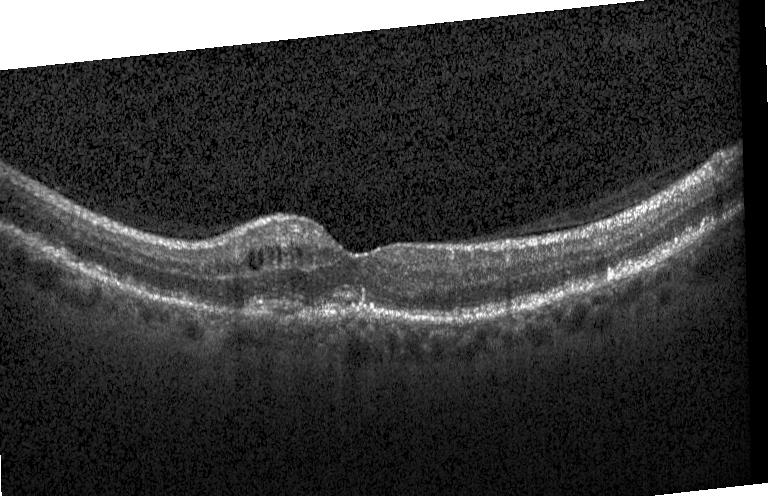

Diagnosis: a choroidal neovascular membrane.